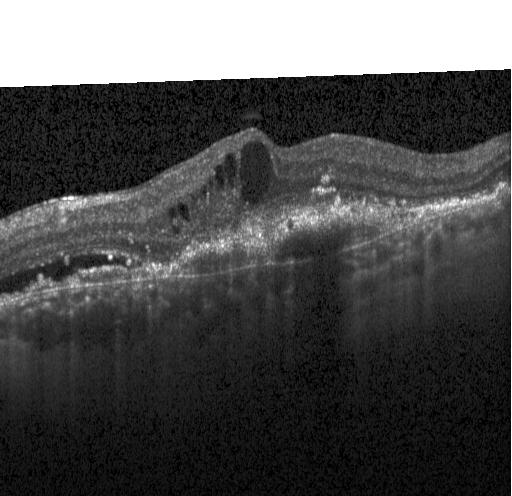
Acquired on a Heidelberg Spectralis. OCT B-scan. Centered on the fovea.
A choroidal neovascular membrane.